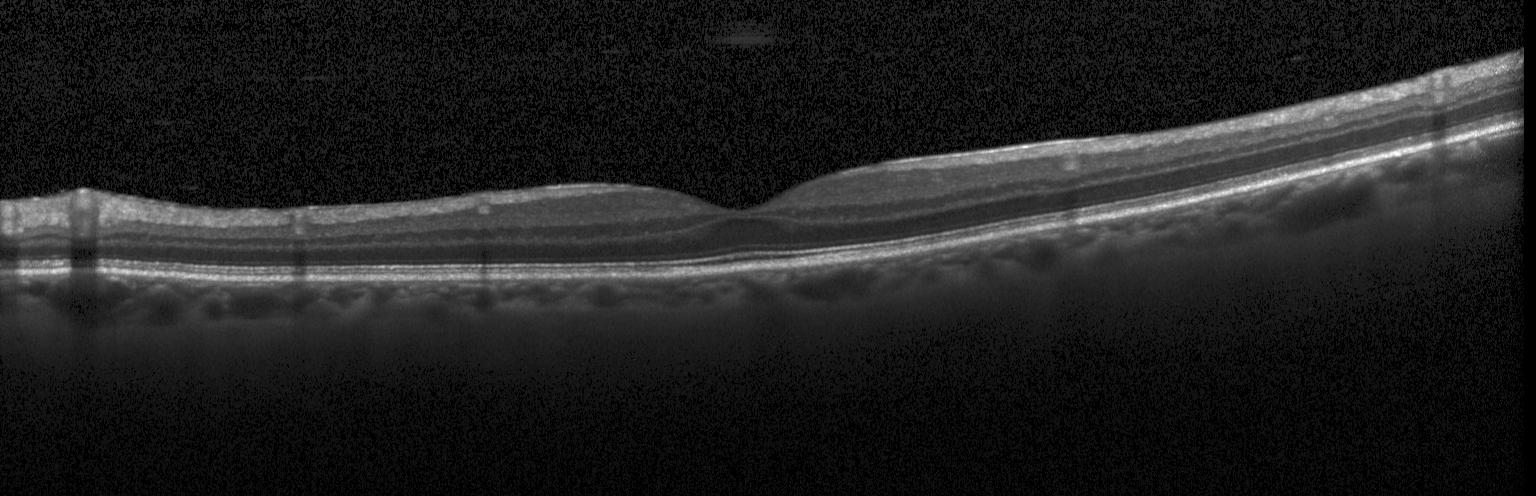 The scan shows no CNV, no DME, and no drusen.